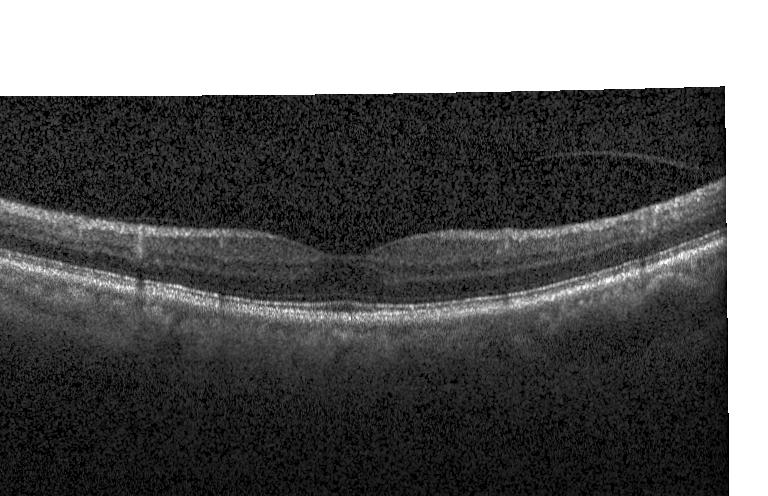

Retinal OCT B-scan. SD-OCT. Macular scan — Finding: no choroidal neovascularization, no diabetic macular edema, and no drusen.